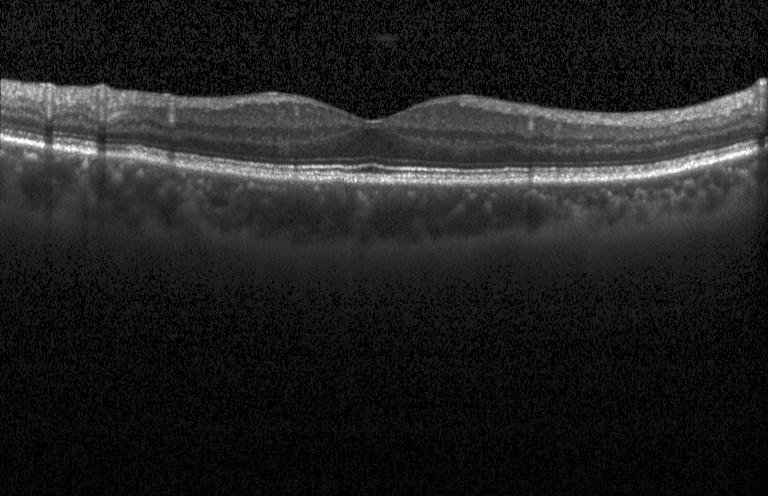 Heidelberg Spectralis. OCT B-scan. Finding: no evidence of choroidal neovascularization, diabetic macular edema, or drusen.